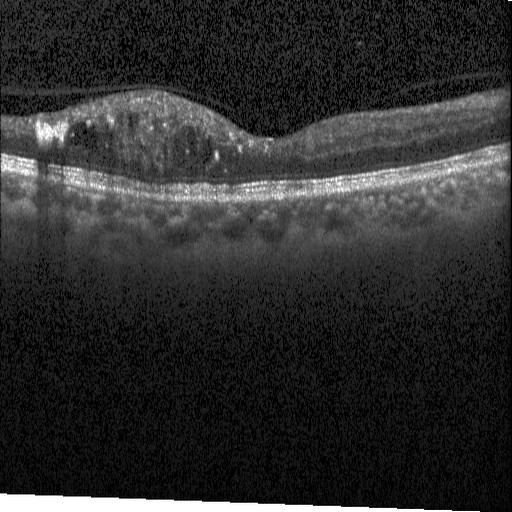 Diagnosis: DME.